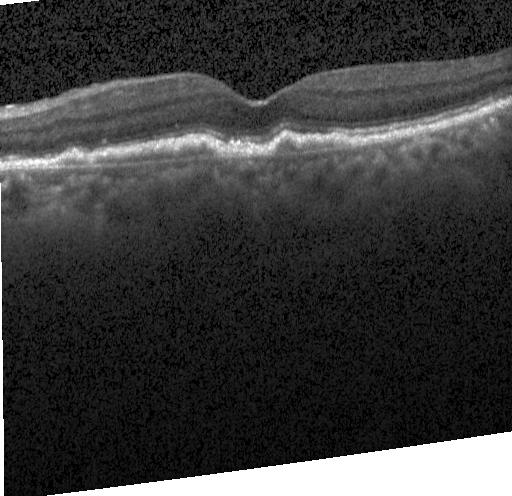
Instrument: Heidelberg Spectralis. Optical coherence tomography B-scan. SD-OCT
Dx: a choroidal neovascular membrane.